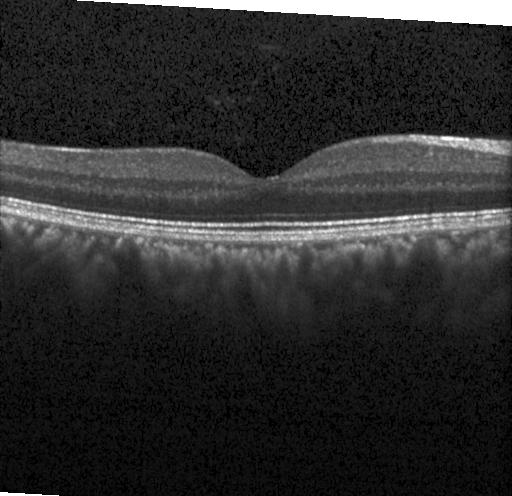

Impression: no choroidal neovascularization, no diabetic macular edema, and no drusen.